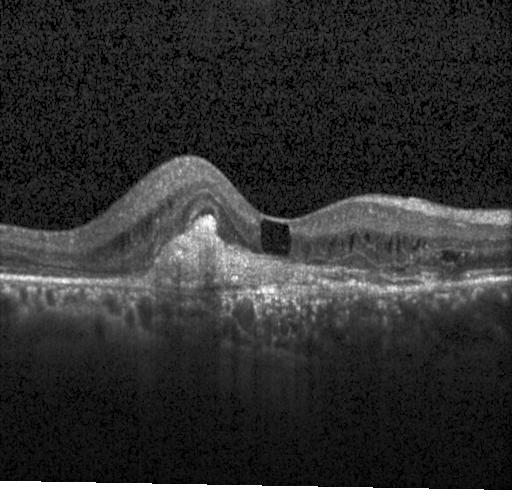 OCT B-scan showing choroidal neovascularization.